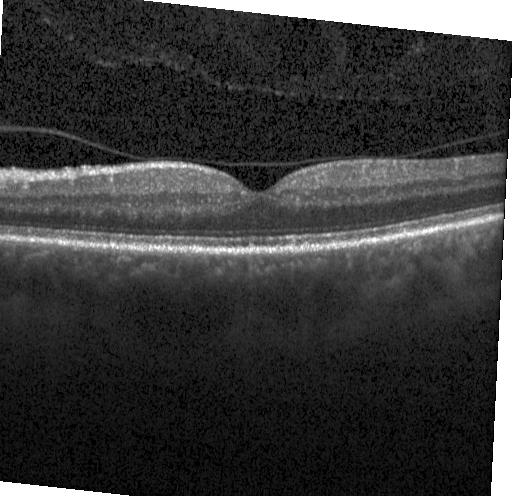 Impression: no choroidal neovascularization, diabetic macular edema, or drusen.